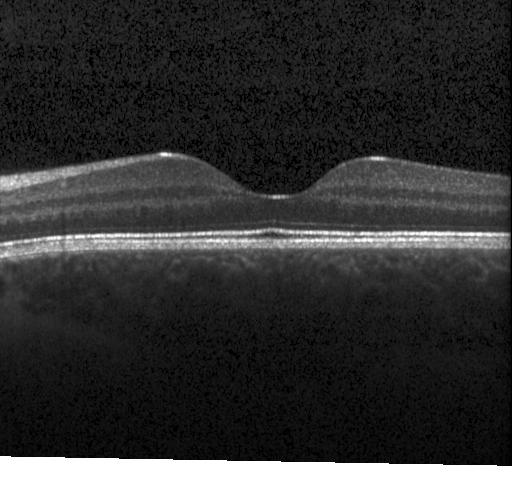
Neither choroidal neovascularization, diabetic macular edema, nor drusen.